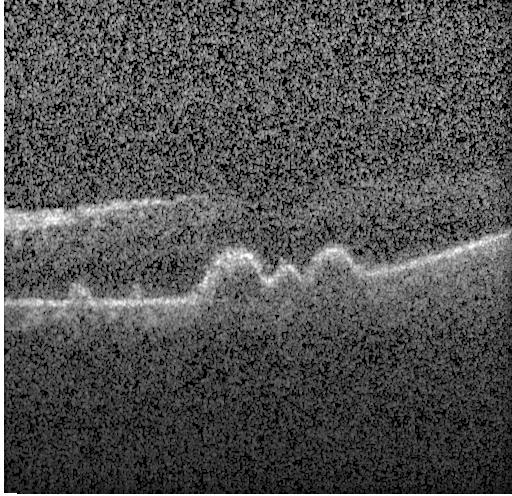

Optical coherence tomography B-scan. Heidelberg Spectralis. Spectral-domain OCT. Fovea-centered
Impression: sub-RPE drusenoid deposits.